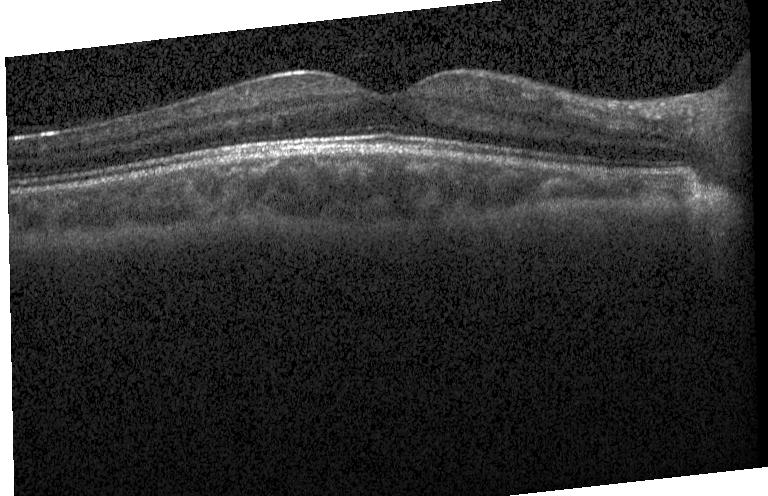
OCT B-scan showing no CNV, DME, or drusen.